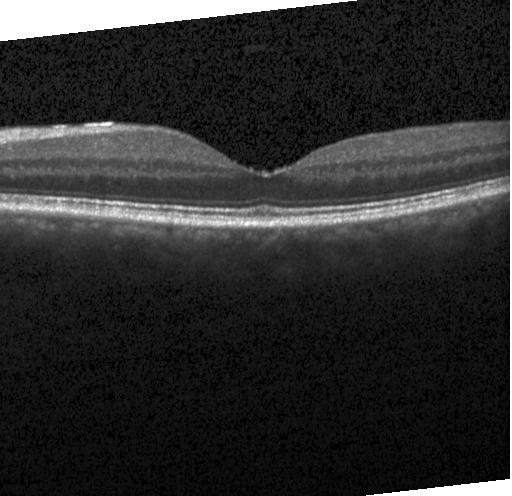 Instrument: Heidelberg Spectralis · through the macula · optical coherence tomography B-scan · spectral-domain OCT — Finding: no evidence of choroidal neovascularization, diabetic macular edema, or drusen.